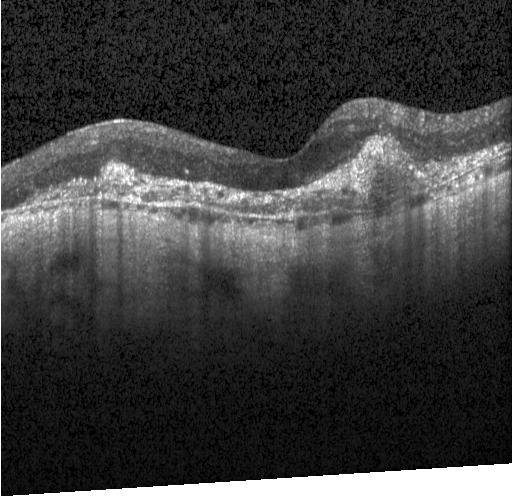
Diagnosis: a choroidal neovascular membrane.